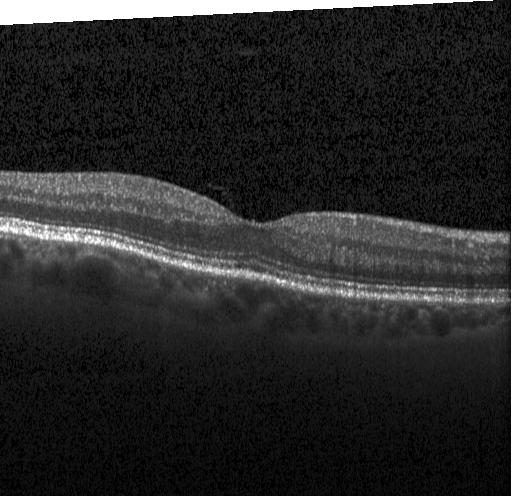

OCT line scan. Centered on the fovea
Impression: no evidence of choroidal neovascularization, diabetic macular edema, or drusen.